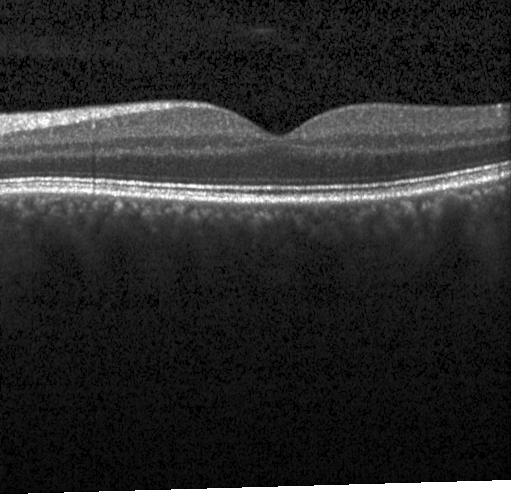
Acquired on a Heidelberg Spectralis, centered on the fovea, OCT line scan. Finding: no choroidal neovascularization, no diabetic macular edema, and no drusen.